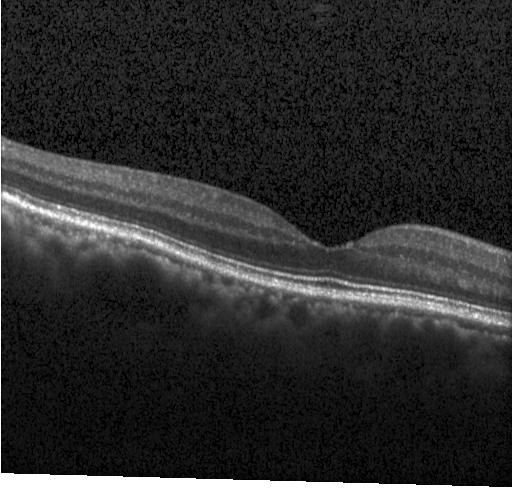

Finding: no evidence of choroidal neovascularization, diabetic macular edema, or drusen.